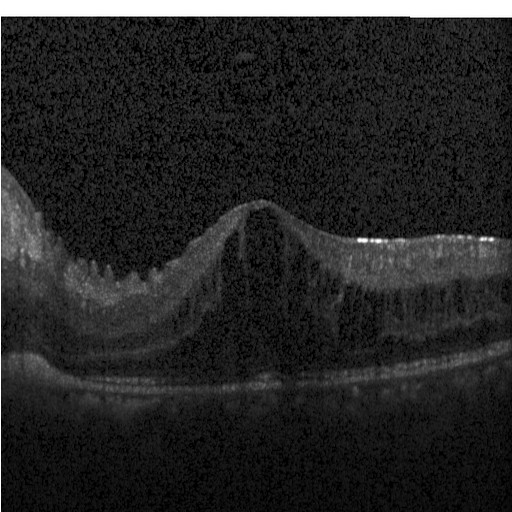
Horizontal scan through the fovea. Optical coherence tomography B-scan — This B-scan demonstrates diabetic macular edema (DME).